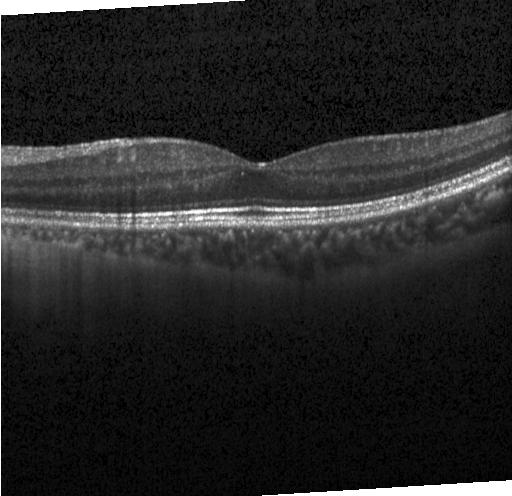 Acquired on a Heidelberg Spectralis · spectral-domain OCT · retinal OCT B-scan. Assessment: no choroidal neovascularization, diabetic macular edema, or drusen.